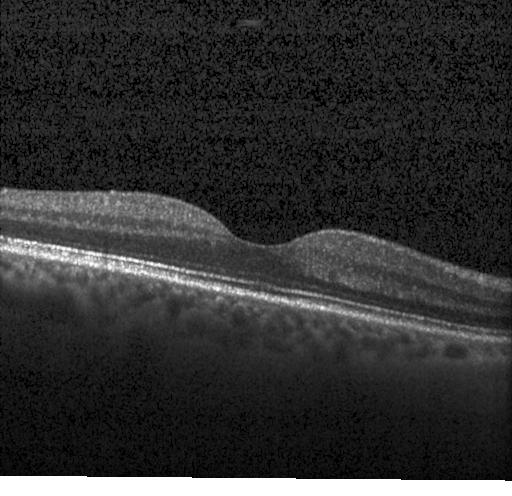

Instrument: Heidelberg Spectralis. Retinal OCT cross-section. No CNV, DME, or drusen.